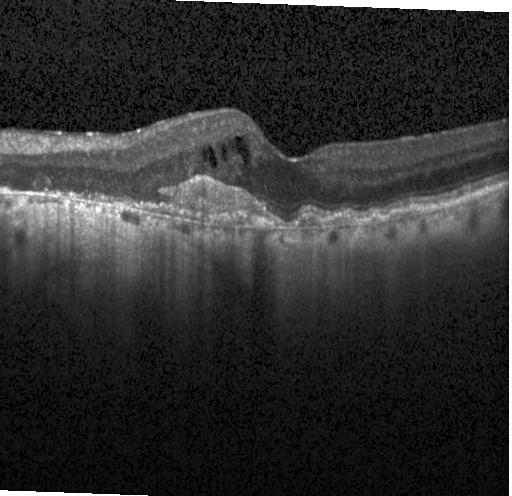

Heidelberg Spectralis; retinal OCT B-scan
Finding: choroidal neovascularization.